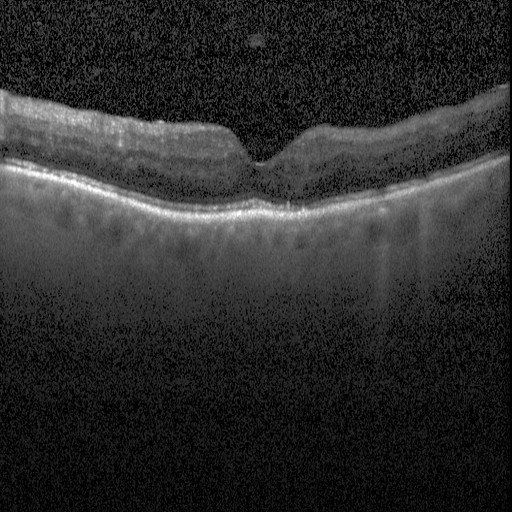

OCT B-scan, instrument: Heidelberg Spectralis, fovea-centered, SD-OCT
Finding: DME.